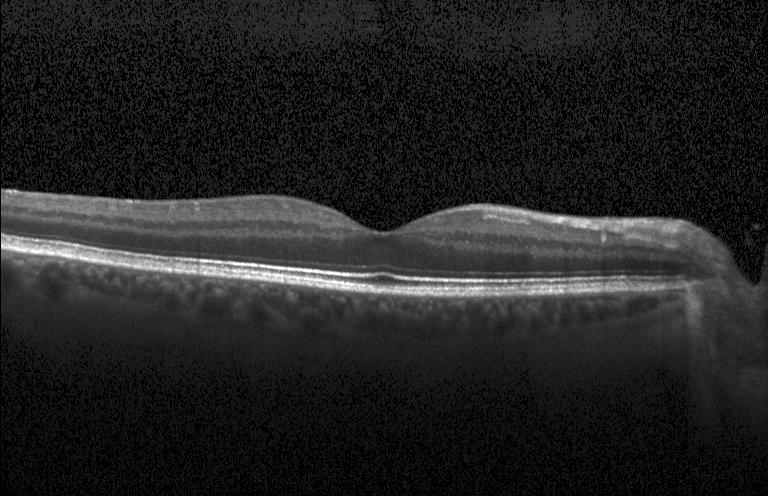 Acquired on a Heidelberg Spectralis. Optical coherence tomography scan. Spectral-domain OCT. Fovea-centered.
Finding: no choroidal neovascularization, no diabetic macular edema, and no drusen.